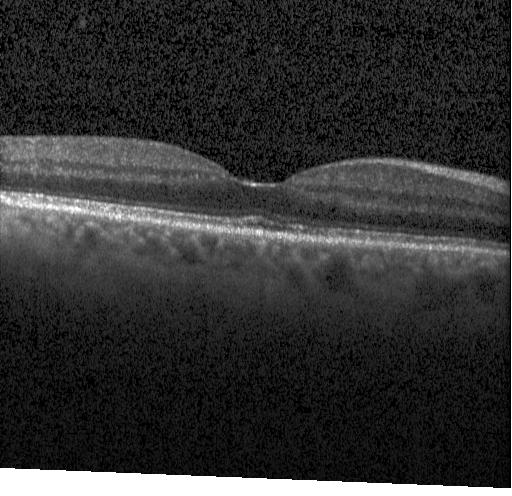 Retinal OCT cross-section showing no choroidal neovascularization, no diabetic macular edema, and no drusen.